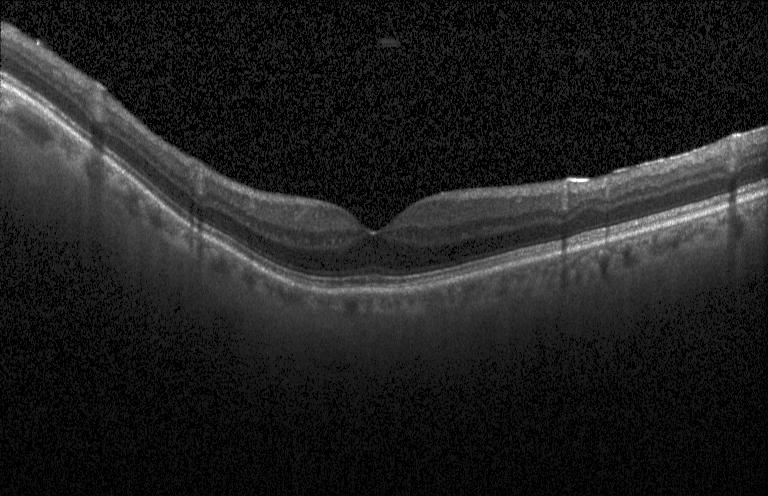
Diagnosis: no evidence of choroidal neovascularization, diabetic macular edema, or drusen.